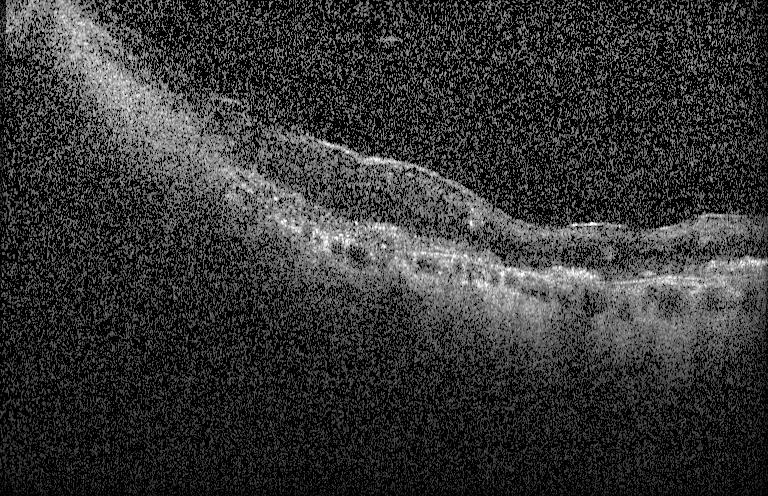 Retinal OCT B-scan. Choroidal neovascularization (CNV).